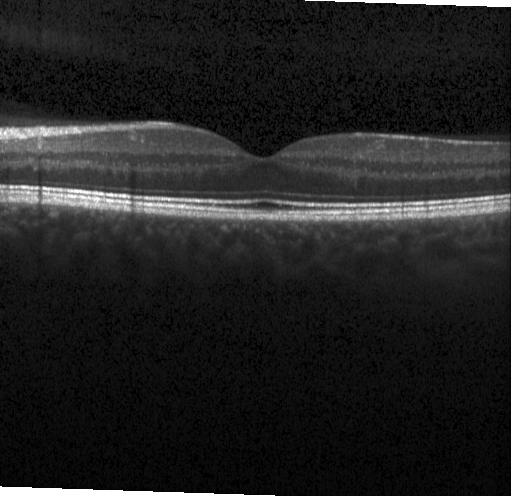
Spectral-domain optical coherence tomography. Instrument: Heidelberg Spectralis. Retinal OCT cross-section — Finding: no evidence of choroidal neovascularization, diabetic macular edema, or drusen.